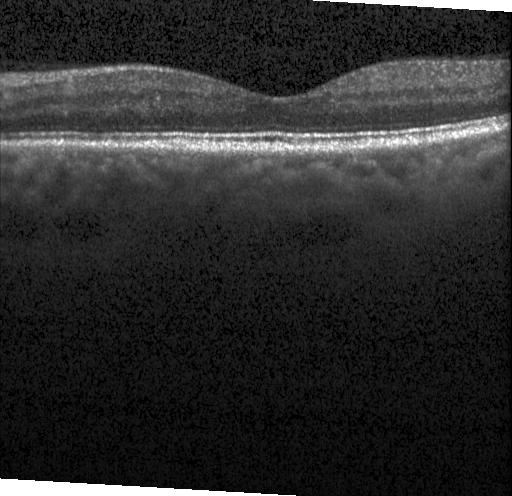 Macular OCT: no choroidal neovascularization, no diabetic macular edema, and no drusen.